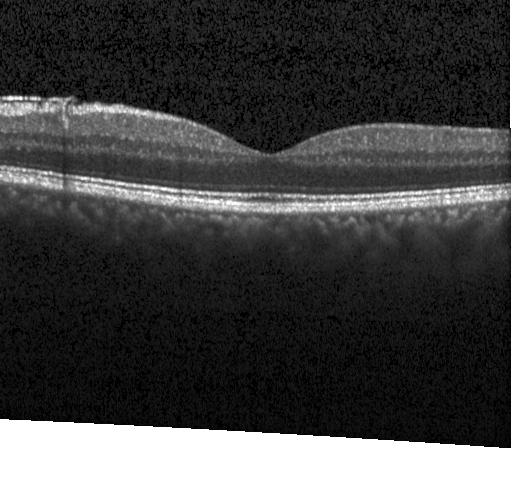 Fovea-centered; OCT line scan — The scan shows neither CNV, DME, nor drusen.